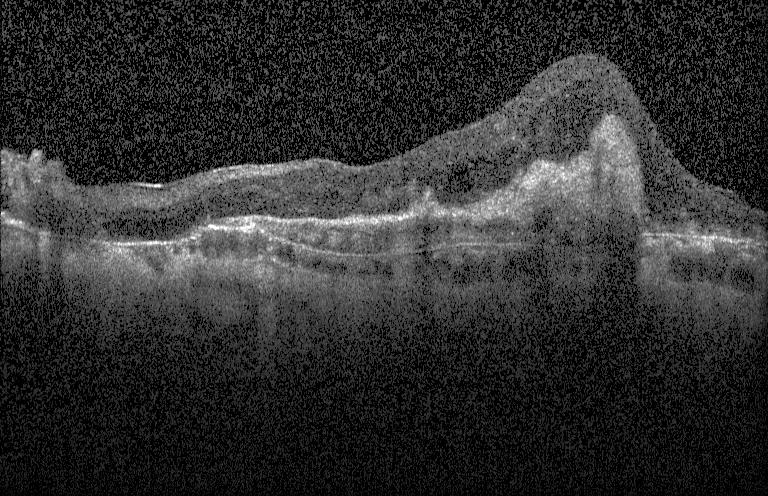 OCT B-scan showing choroidal neovascularization (CNV).